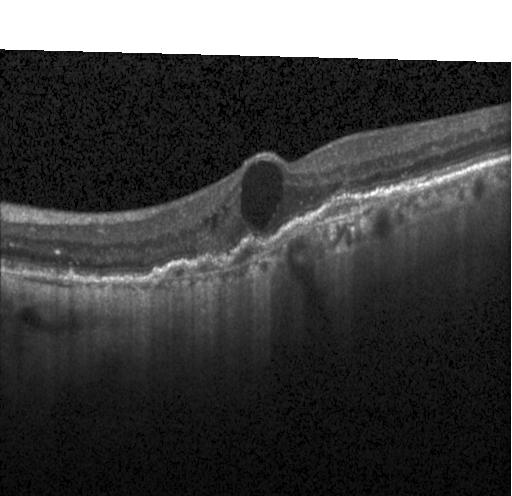

Optical coherence tomography B-scan · spectral-domain optical coherence tomography · horizontal scan through the fovea · Heidelberg Spectralis.
CNV.